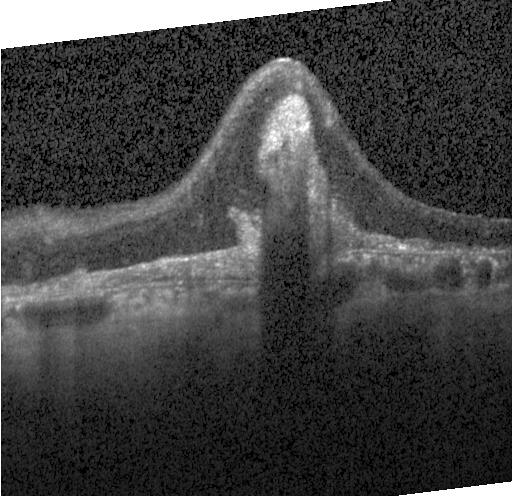 OCT B-scan showing choroidal neovascularization.